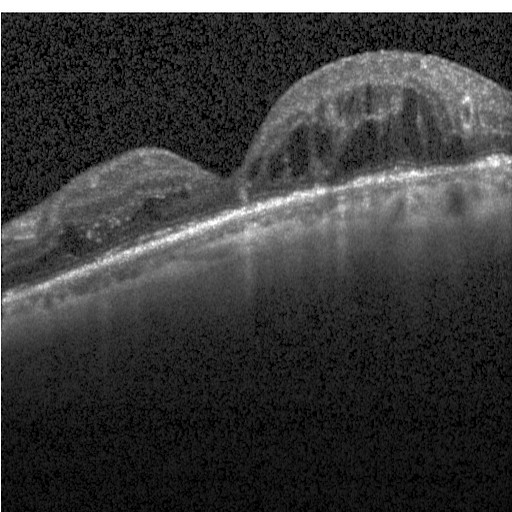
OCT scan showing diabetic macular edema (DME).